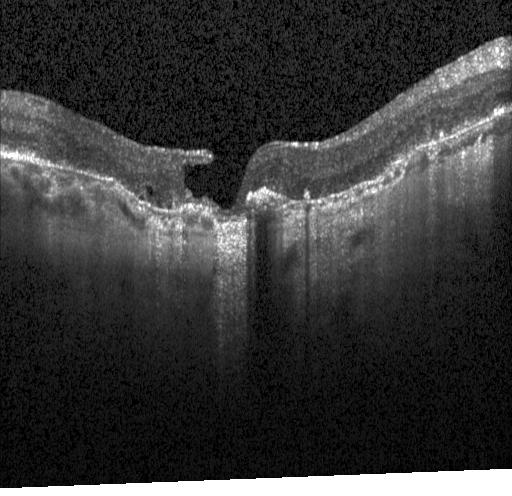

Centered on the fovea · retinal OCT cross-section.
The scan shows choroidal neovascularization (CNV).